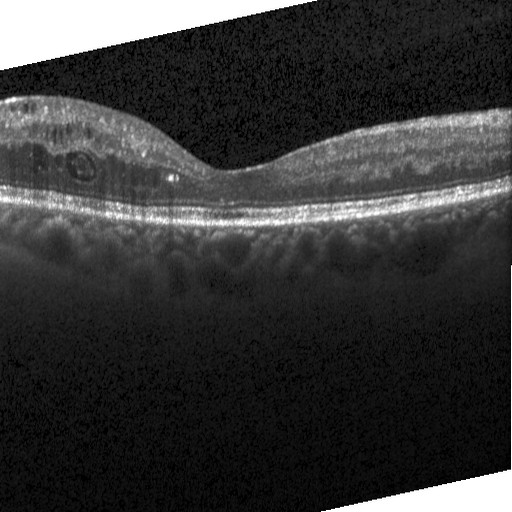

Optical coherence tomography B-scan. Finding: diabetic macular edema.